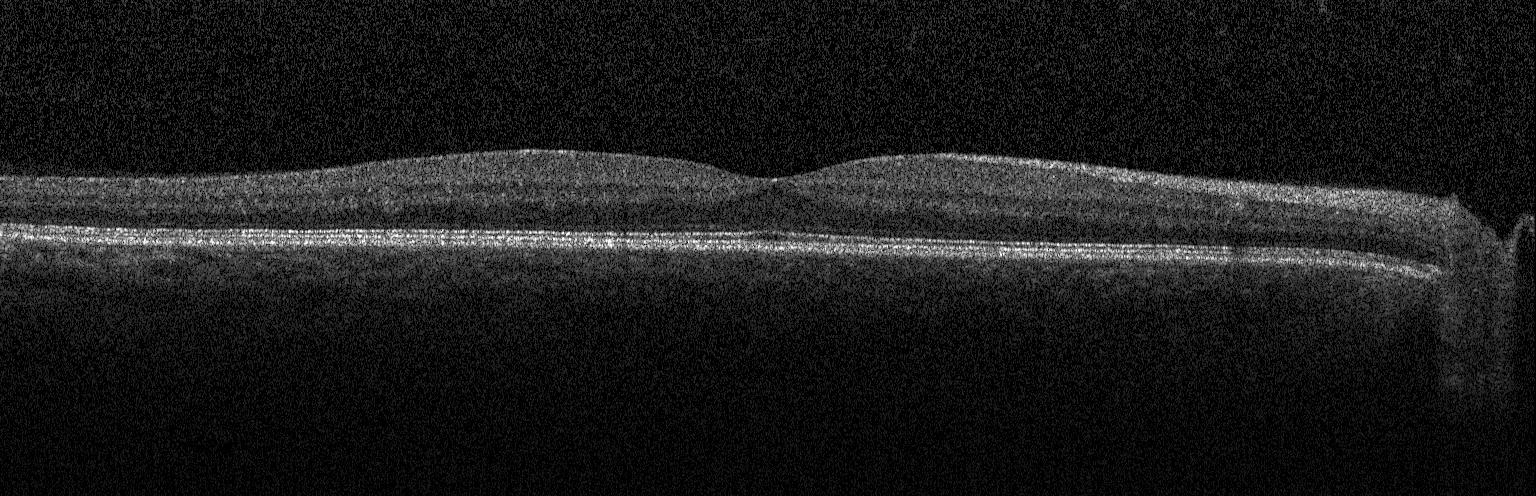 Macular OCT: no choroidal neovascularization, diabetic macular edema, or drusen.